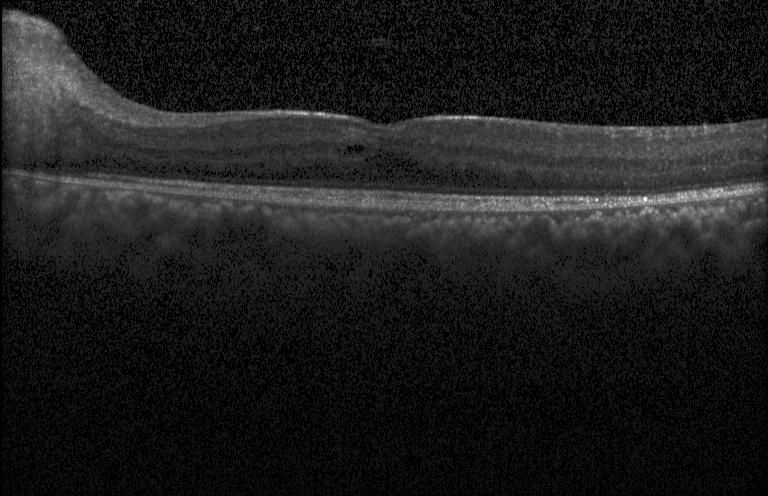
Impression: diabetic macular edema.